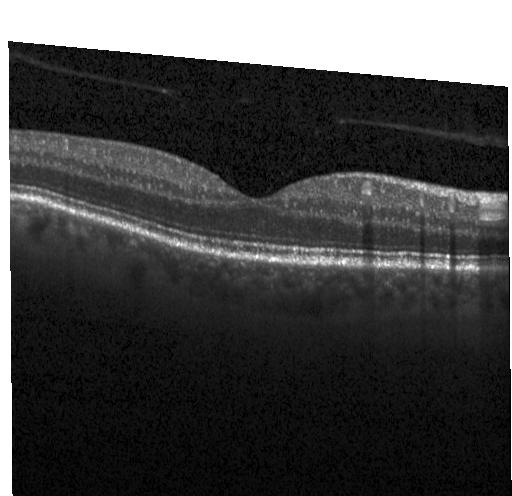

Macular OCT: no choroidal neovascularization, diabetic macular edema, or drusen.